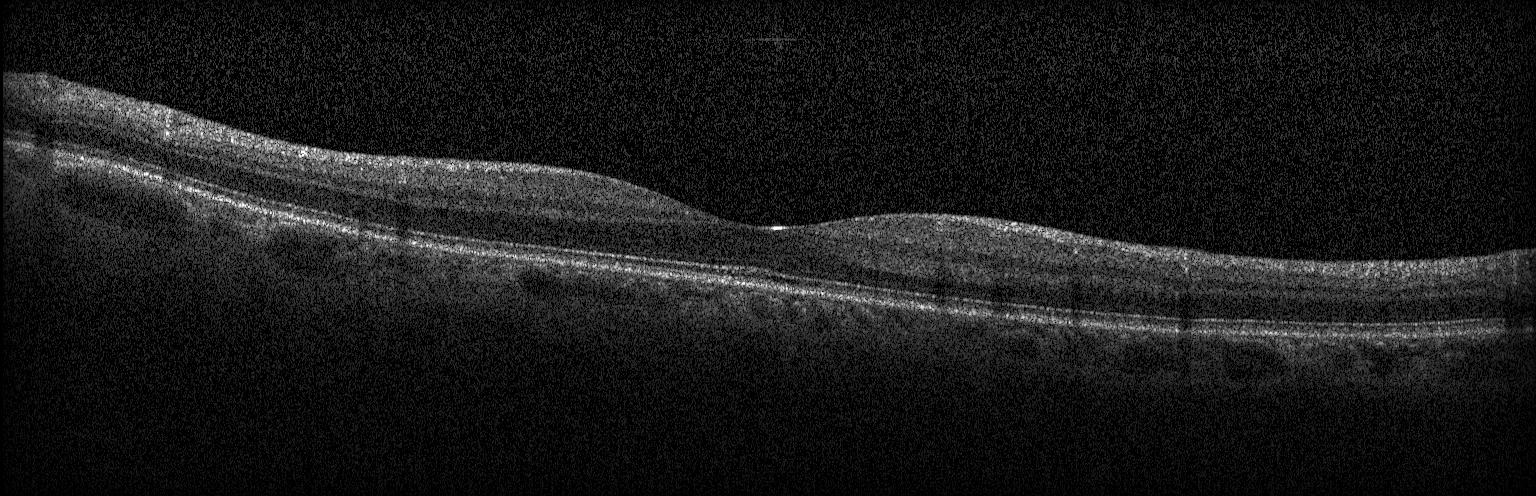 Assessment: neither CNV, DME, nor drusen.